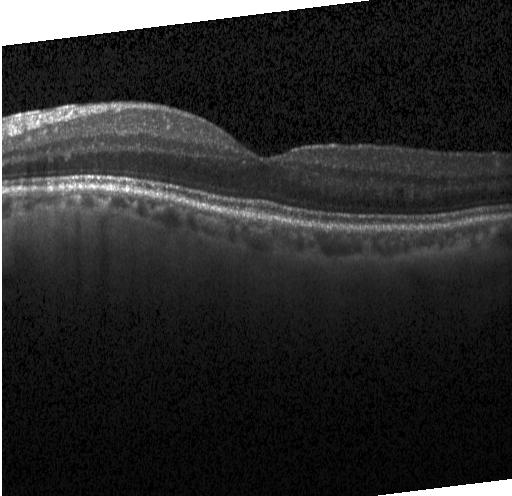

OCT B-scan. Heidelberg Spectralis OCT system — Neither choroidal neovascularization, diabetic macular edema, nor drusen.